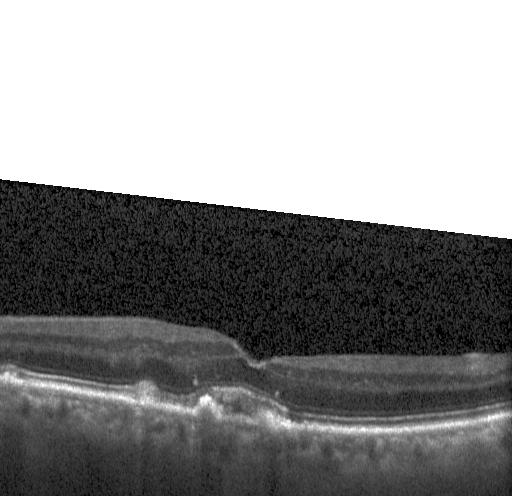

This B-scan demonstrates a choroidal neovascular membrane.